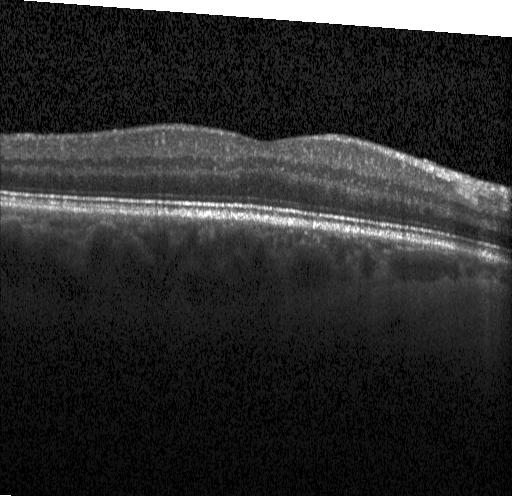 OCT B-scan showing neither choroidal neovascularization, diabetic macular edema, nor drusen.